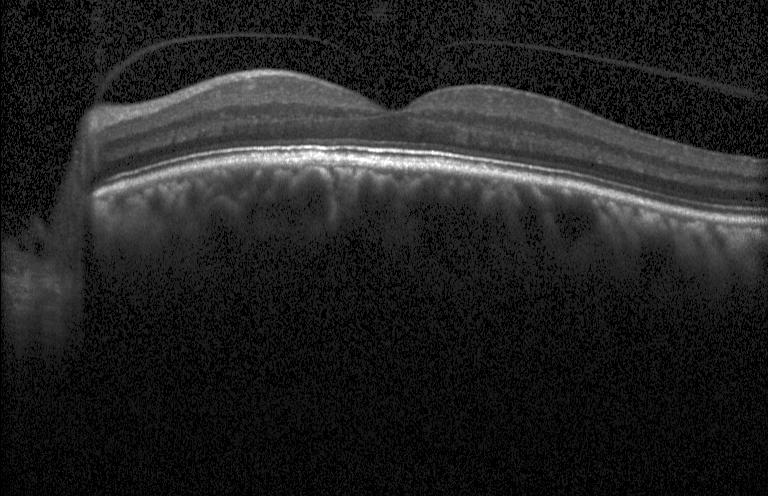

The scan shows no choroidal neovascularization, no diabetic macular edema, and no drusen.